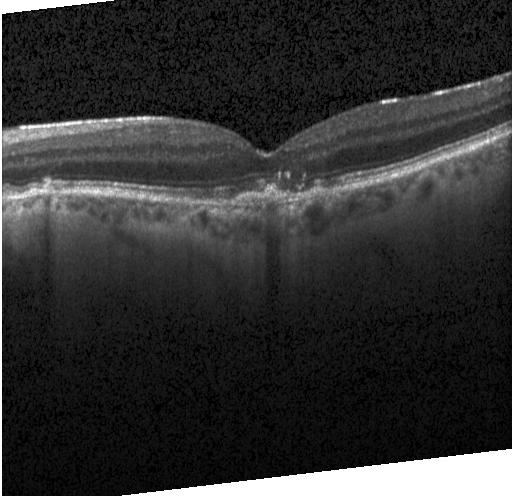
Impression: choroidal neovascularization.